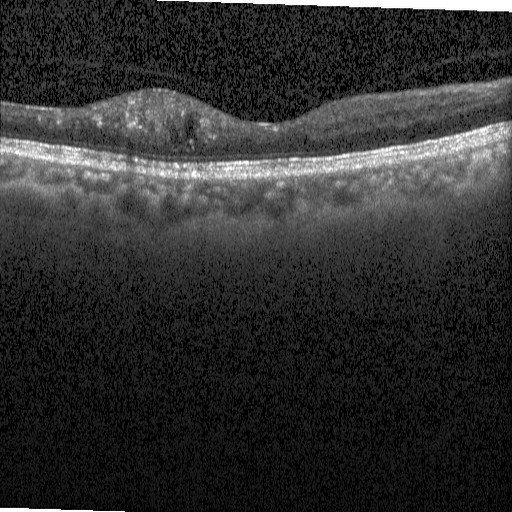

Retinal OCT B-scan
Assessment: diabetic macular edema (DME).